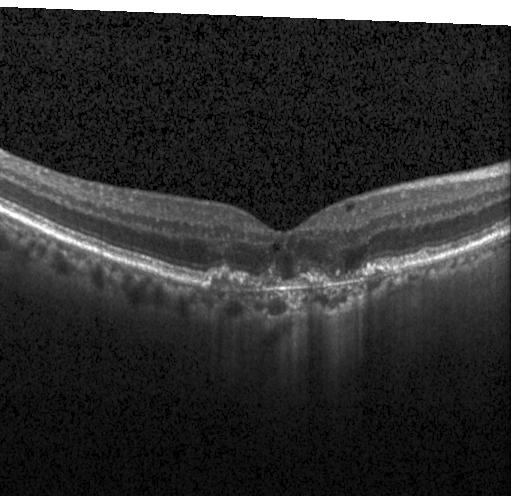
Retinal OCT B-scan
Diagnosis: a choroidal neovascular membrane.